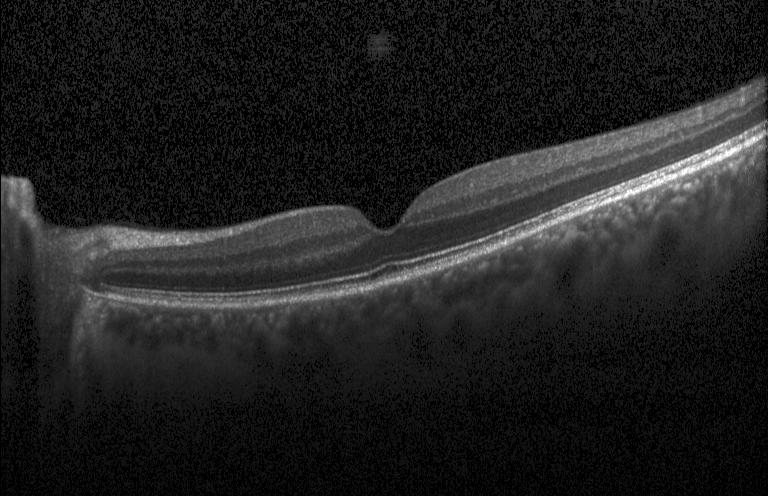 Instrument: Heidelberg Spectralis. Retinal OCT cross-section. Centered on the fovea. SD-OCT. Finding: no CNV, no DME, and no drusen.